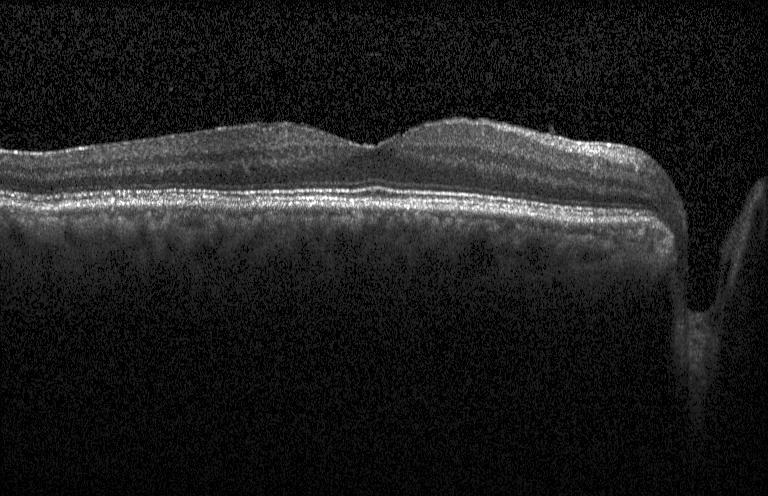

OCT B-scan, through the macula, instrument: Heidelberg Spectralis, SD-OCT — Impression: neither choroidal neovascularization, diabetic macular edema, nor drusen.